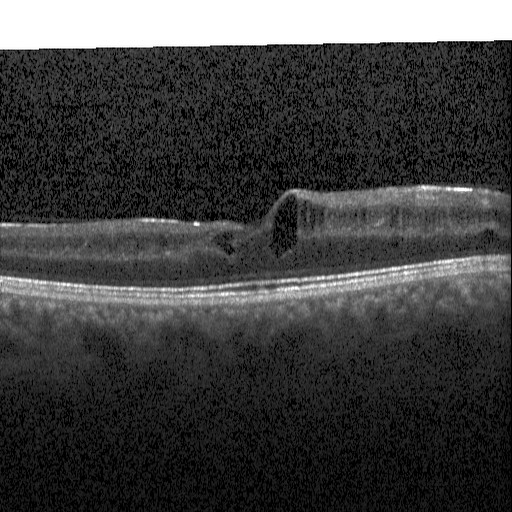 Optical coherence tomography B-scan; acquired on a Heidelberg Spectralis — Diagnosis: diabetic macular edema.